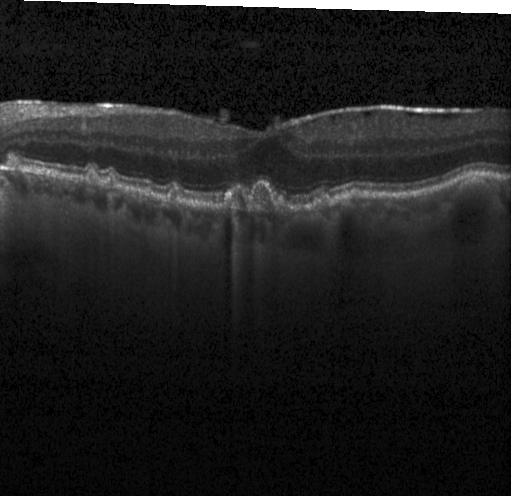
Retinal OCT cross-section showing multiple drusen.